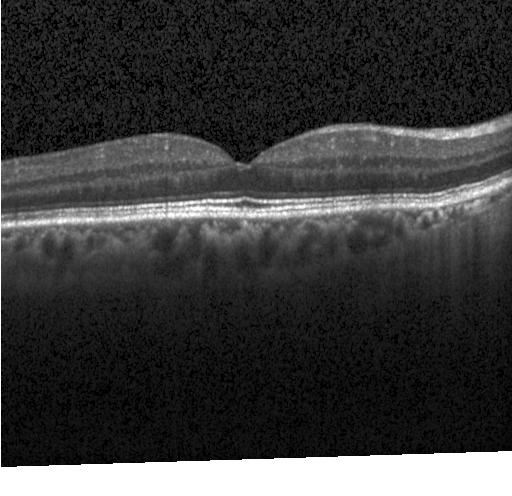 OCT finding: neither choroidal neovascularization, diabetic macular edema, nor drusen.